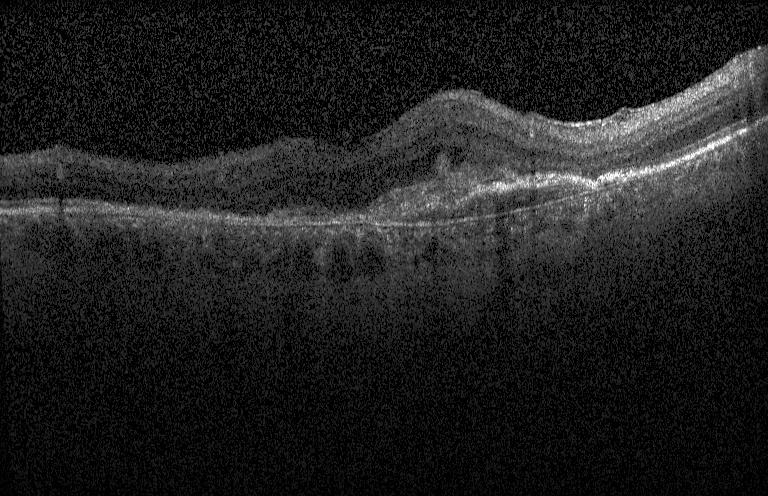 SD-OCT. Through the macula. Heidelberg Spectralis. Optical coherence tomography B-scan. The scan shows CNV.